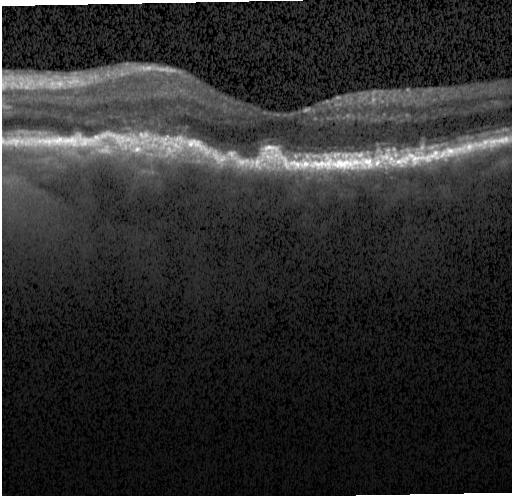
Instrument: Heidelberg Spectralis. OCT line scan. SD-OCT. Fovea-centered
The scan shows choroidal neovascularization.